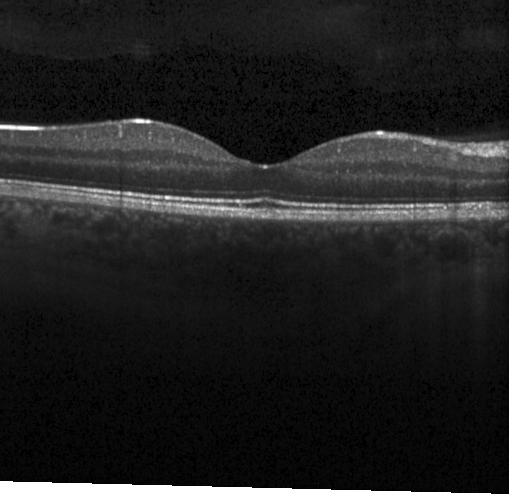
Diagnosis: neither choroidal neovascularization, diabetic macular edema, nor drusen.